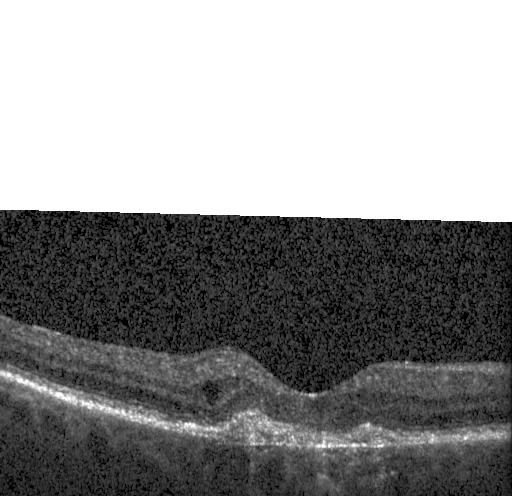 Heidelberg Spectralis OCT system; OCT B-scan
Choroidal neovascularization.